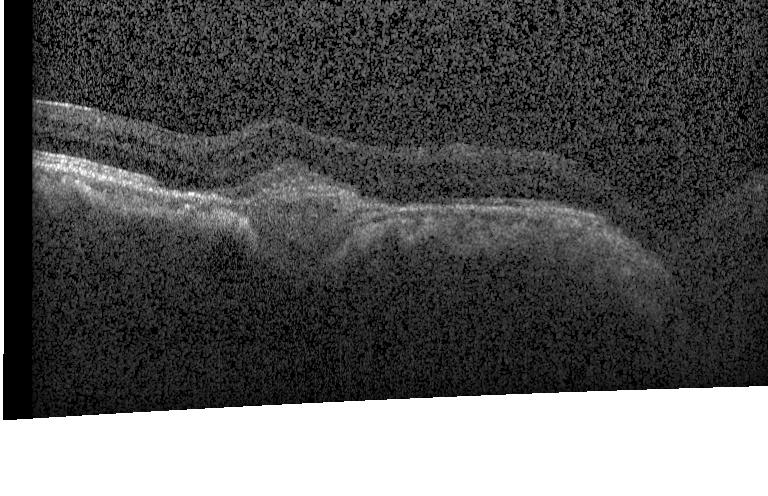

Impression: choroidal neovascularization.